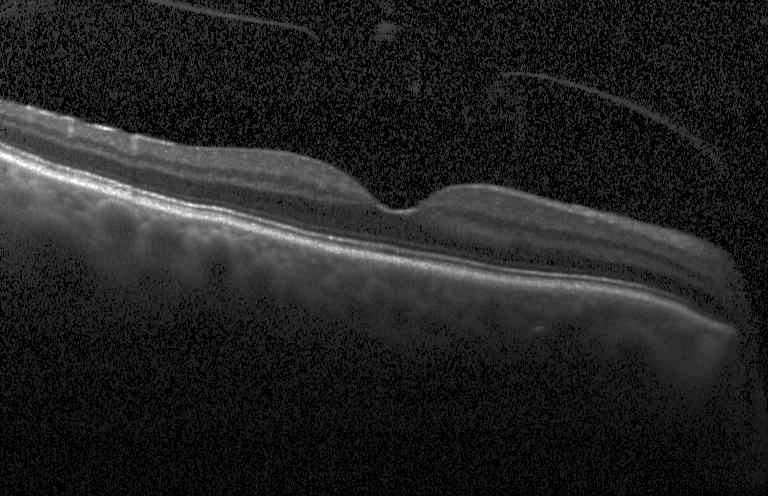
Through the macula · OCT B-scan.
Neither CNV, DME, nor drusen.